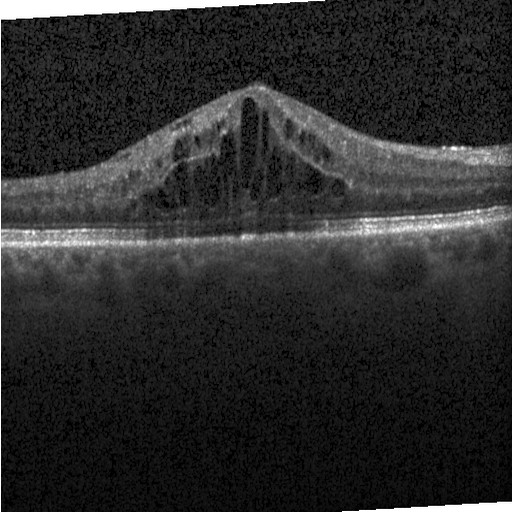
Spectral-domain OCT B-scan: diabetic macular edema.